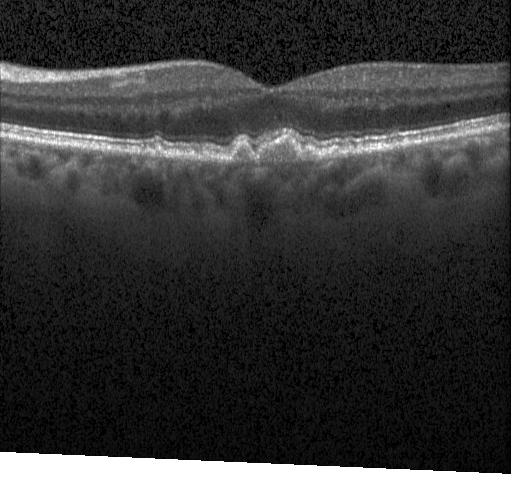

Spectral-domain optical coherence tomography. Horizontal scan through the fovea. OCT line scan
Impression: drusen.